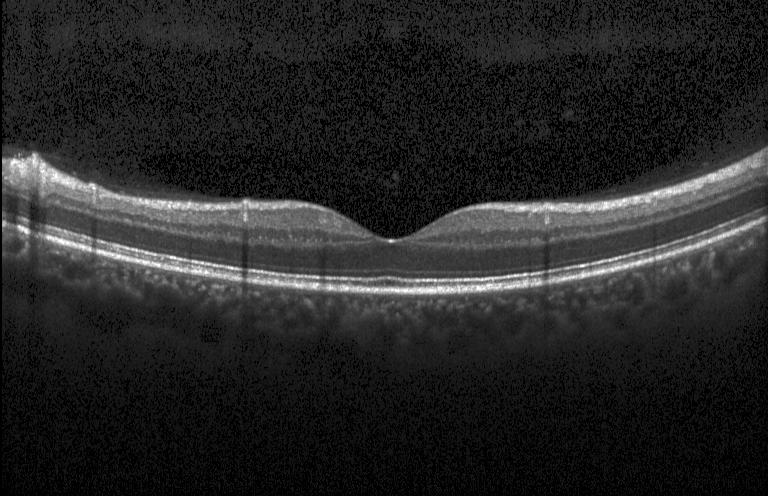
This B-scan demonstrates no evidence of choroidal neovascularization, diabetic macular edema, or drusen.